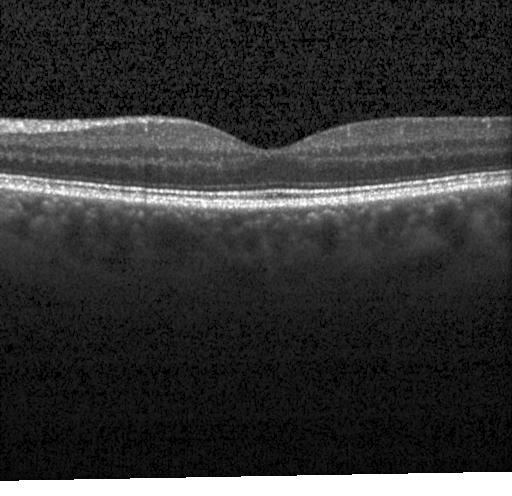 Retinal OCT B-scan; SD-OCT.
Macular OCT: neither choroidal neovascularization, diabetic macular edema, nor drusen.